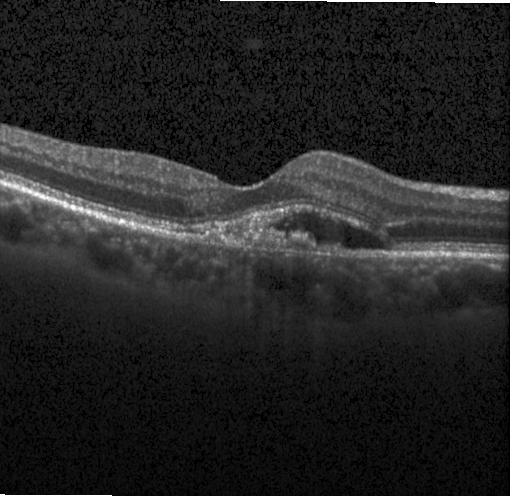 Spectral-domain optical coherence tomography. Optical coherence tomography B-scan. Heidelberg Spectralis — A choroidal neovascular membrane.